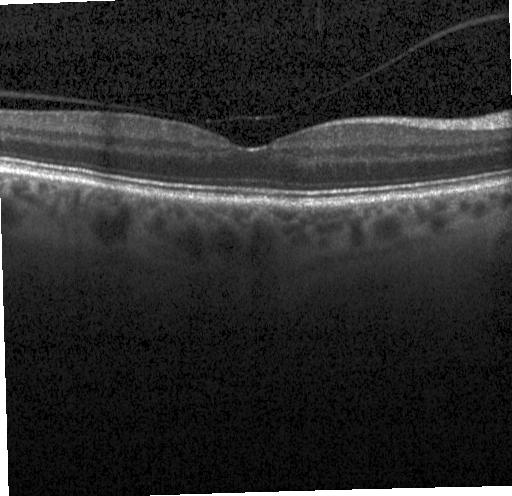 OCT finding: neither choroidal neovascularization, diabetic macular edema, nor drusen.